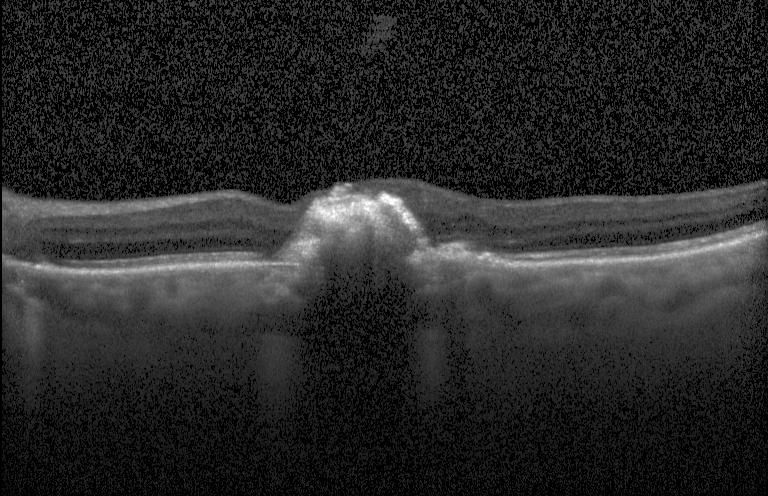

Impression: choroidal neovascularization.